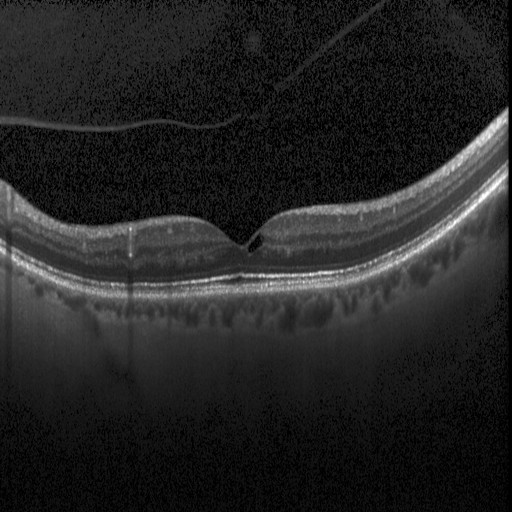
OCT finding: DME.